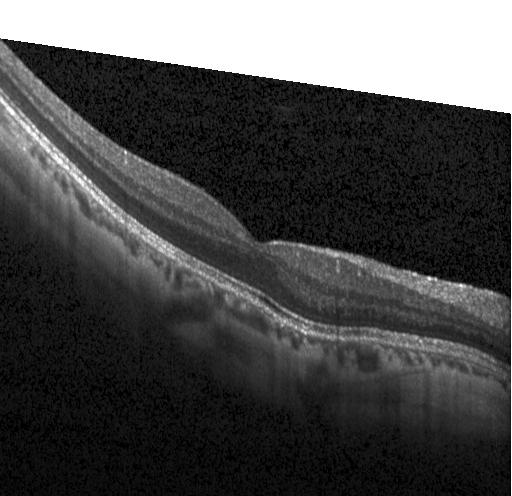
Retinal OCT B-scan · spectral-domain optical coherence tomography · Heidelberg Spectralis — Assessment: no evidence of CNV, DME, or drusen.